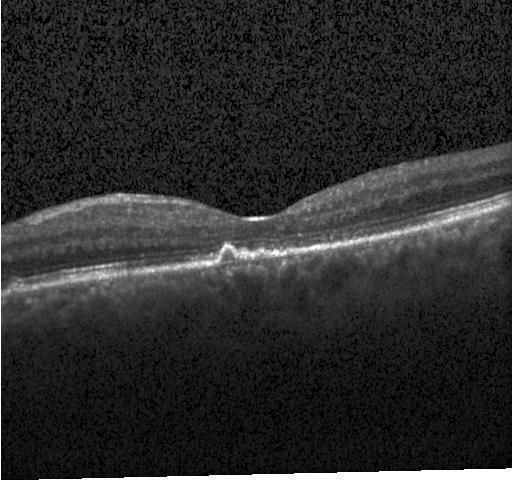
Dx: drusen.